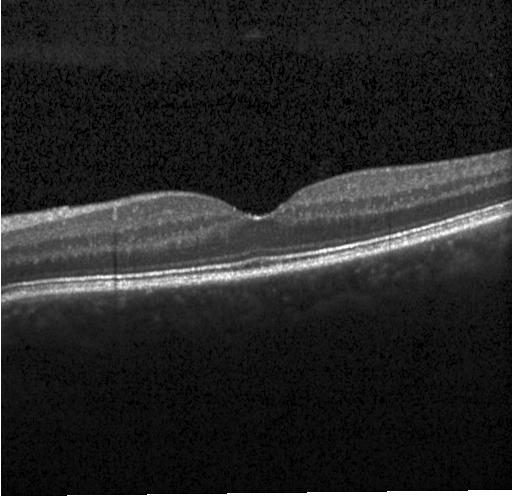 Spectral-domain optical coherence tomography; OCT line scan.
Finding: no evidence of choroidal neovascularization, diabetic macular edema, or drusen.